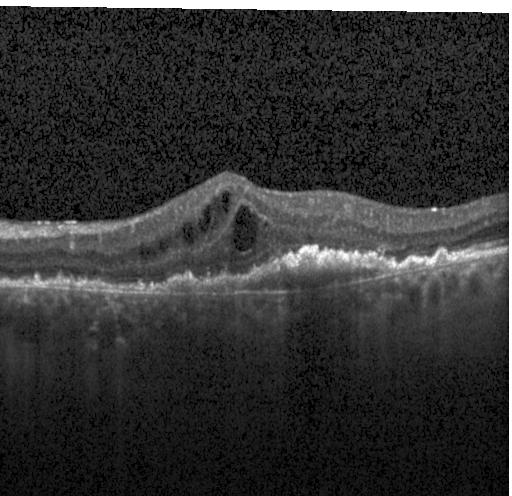
A choroidal neovascular membrane.